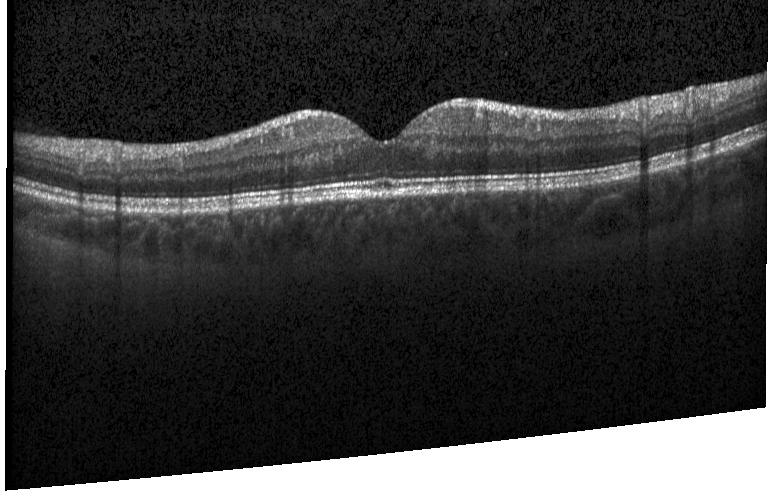
This B-scan demonstrates no choroidal neovascularization, no diabetic macular edema, and no drusen.